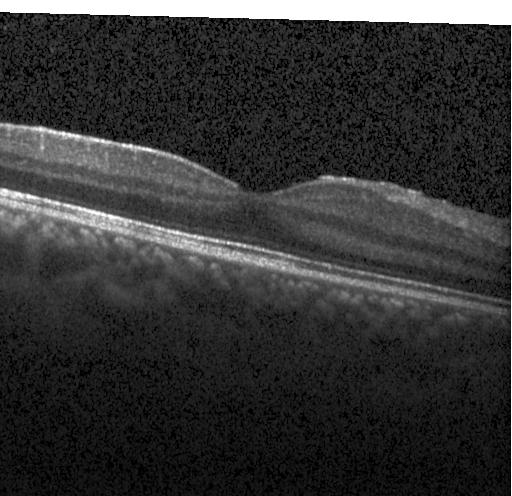 Impression: no choroidal neovascularization, no diabetic macular edema, and no drusen.